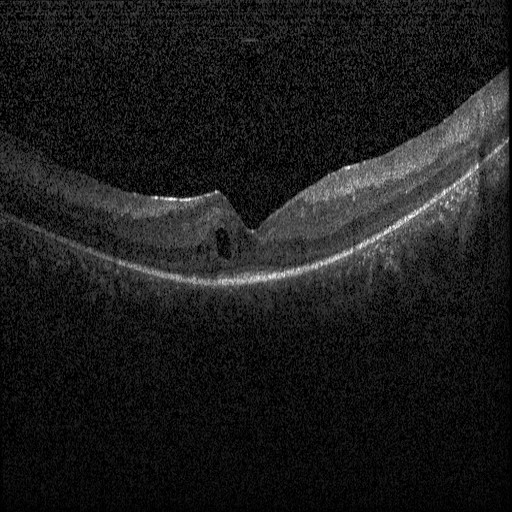

Retinal OCT B-scan, SD-OCT, centered on the fovea.
Assessment: diabetic macular edema.